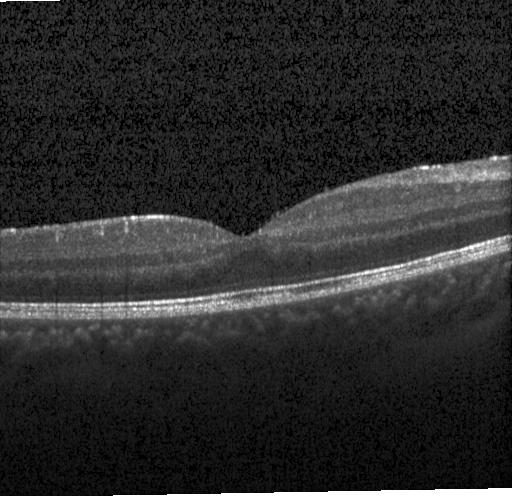 Retinal OCT B-scan; Heidelberg Spectralis; SD-OCT — Impression: no choroidal neovascularization, no diabetic macular edema, and no drusen.